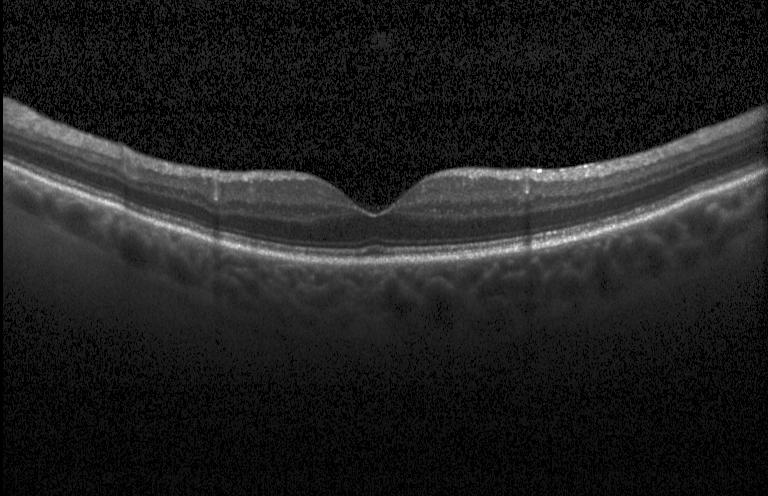

Retinal OCT B-scan. Acquired on a Heidelberg Spectralis.
The scan shows no evidence of choroidal neovascularization, diabetic macular edema, or drusen.